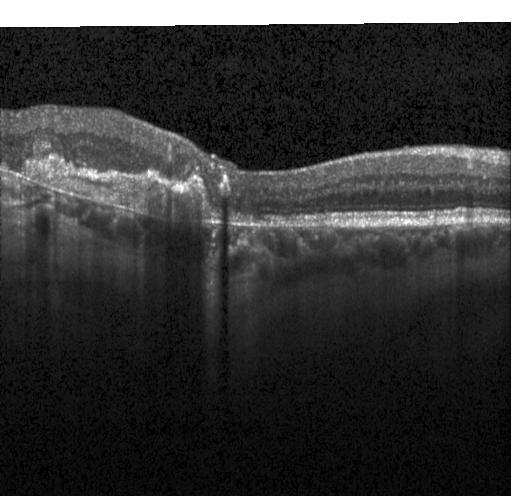

Finding: a choroidal neovascular membrane.